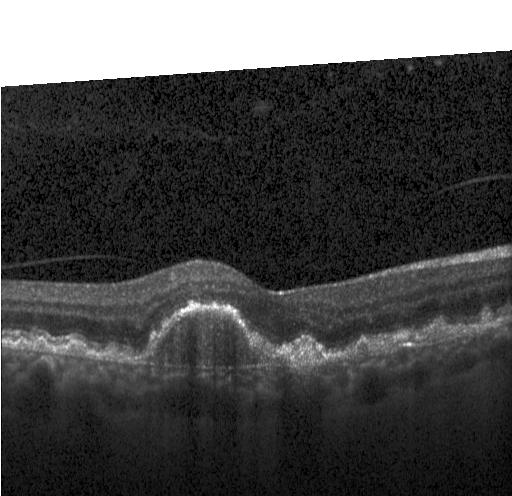
Optical coherence tomography B-scan — Impression: choroidal neovascularization.